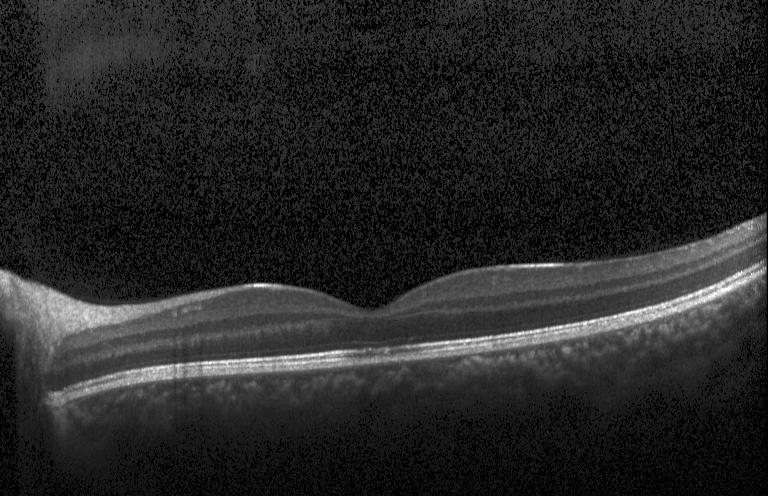

Optical coherence tomography B-scan; centered on the fovea; spectral-domain OCT
Impression: no choroidal neovascularization, no diabetic macular edema, and no drusen.